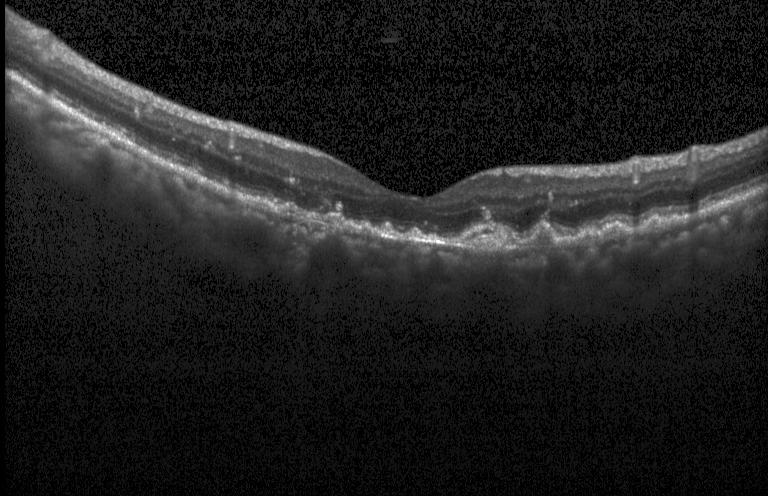

Spectral-domain optical coherence tomography; horizontal scan through the fovea; retinal OCT B-scan; acquired on a Heidelberg Spectralis.
Impression: a choroidal neovascular membrane.